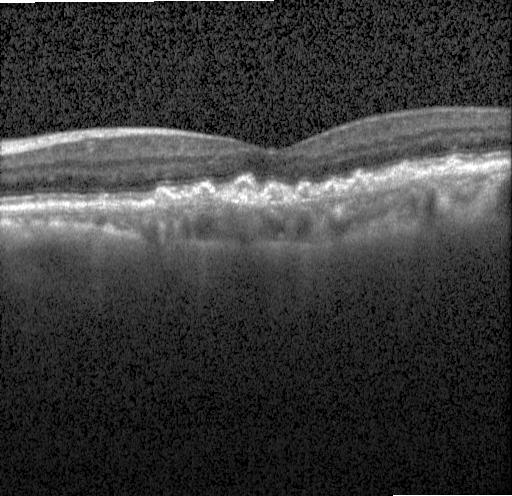

This B-scan demonstrates sub-RPE drusenoid deposits.